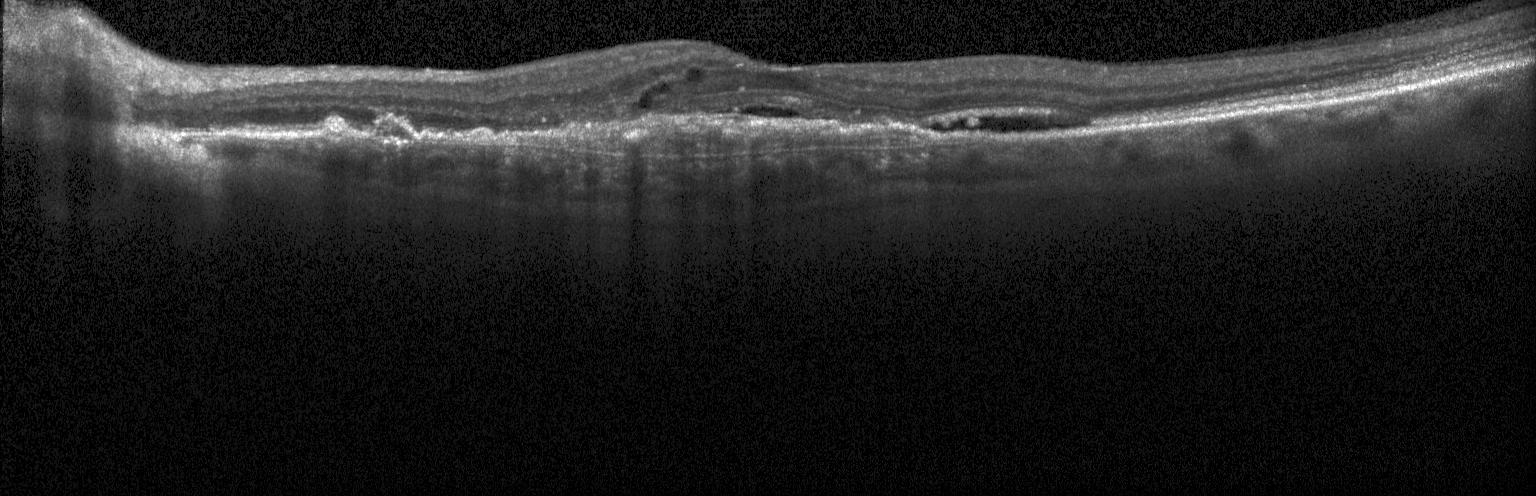 Diagnosis: a choroidal neovascular membrane.